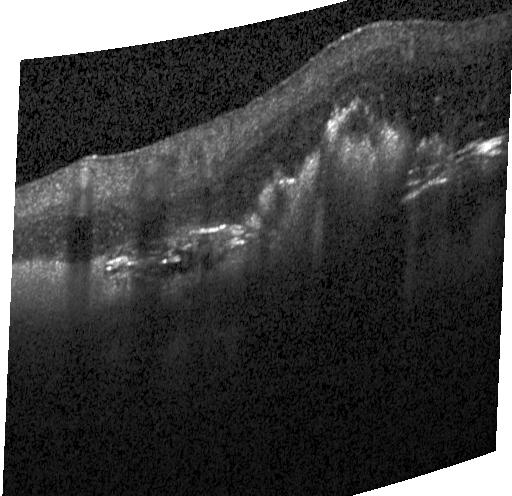 Macular scan, optical coherence tomography scan, instrument: Heidelberg Spectralis, spectral-domain optical coherence tomography.
The scan shows CNV.